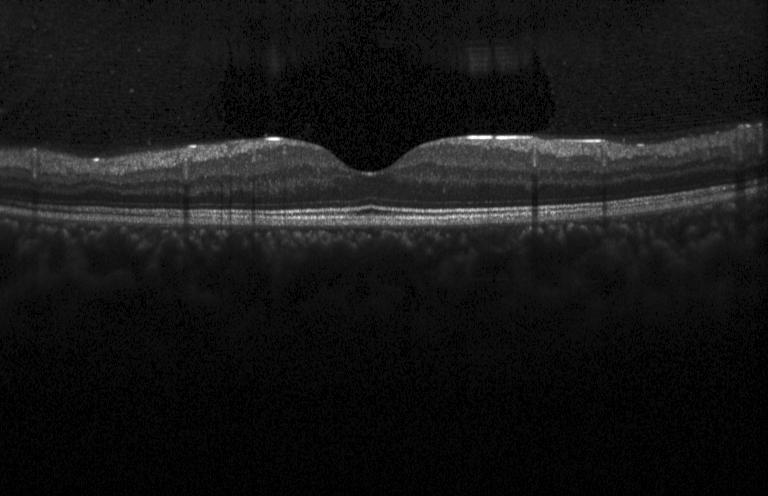 OCT B-scan. SD-OCT — The scan shows no choroidal neovascularization, diabetic macular edema, or drusen.